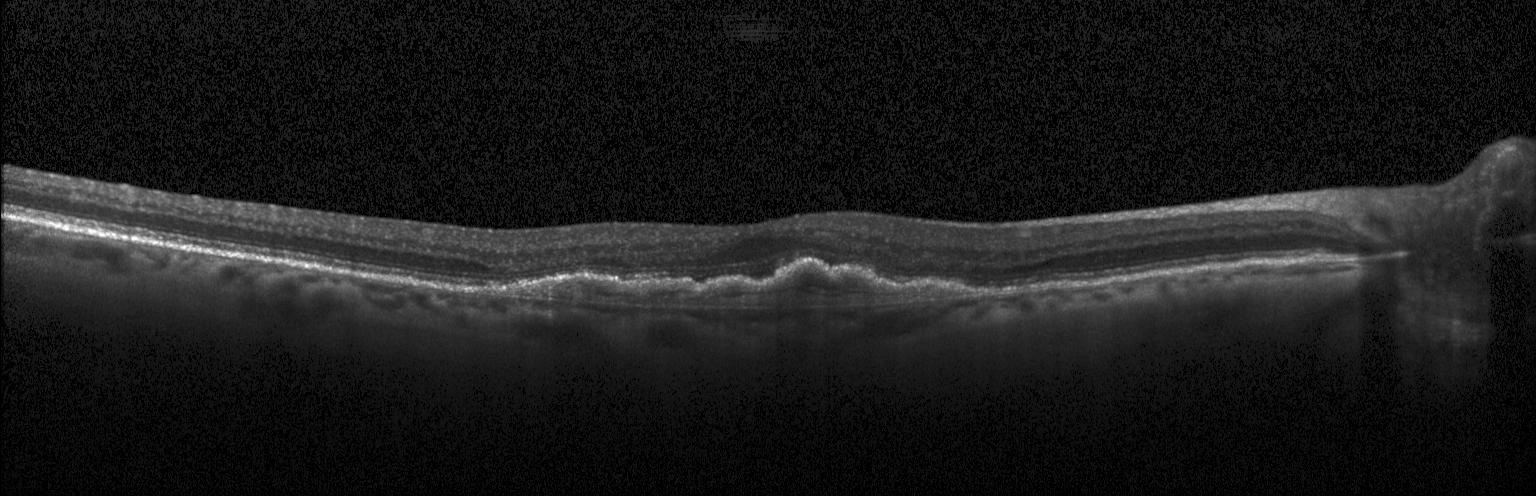
Diagnosis: CNV.